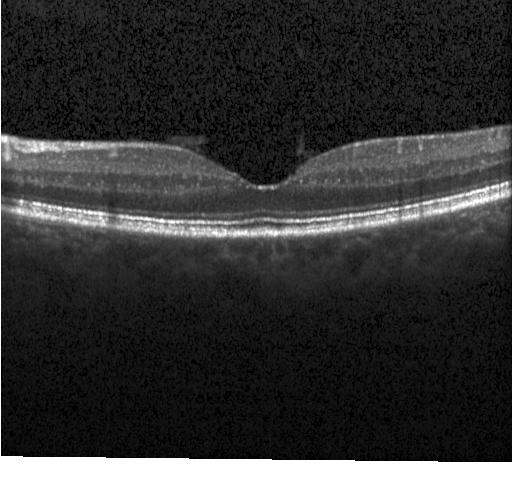

OCT scan showing no CNV, DME, or drusen.